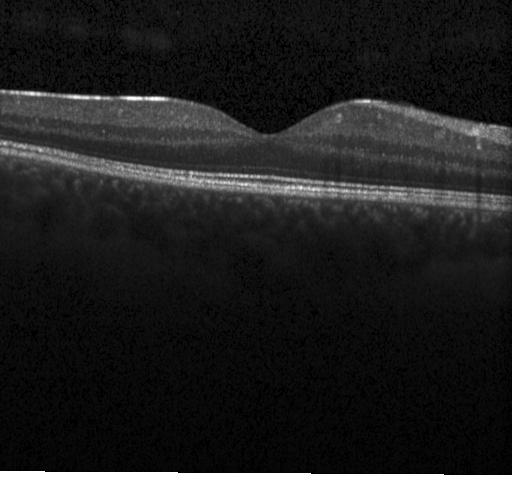
Macular scan. Optical coherence tomography scan. Spectral-domain OCT.
Finding: no CNV, no DME, and no drusen.